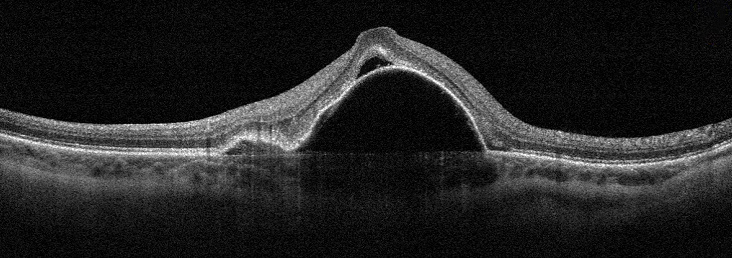
Through the macula · retinal OCT B-scan · Optovue Avanti RTVue XR — Macular OCT: age-related macular degeneration.